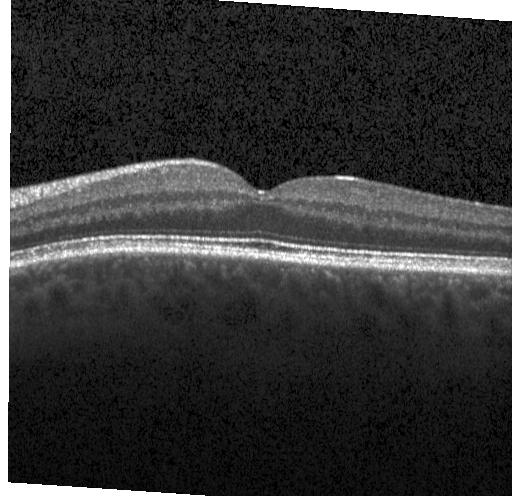 The scan shows neither choroidal neovascularization, diabetic macular edema, nor drusen.